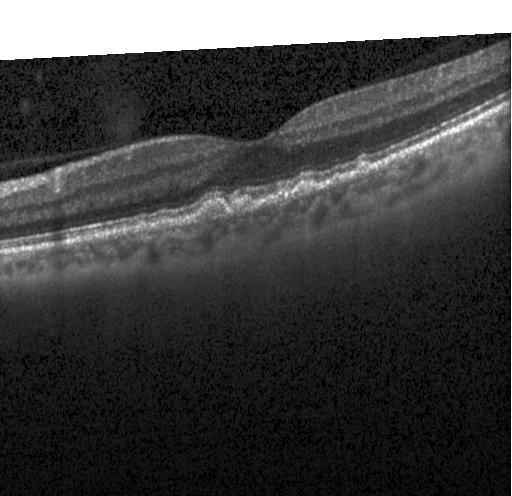

Assessment: multiple drusen.